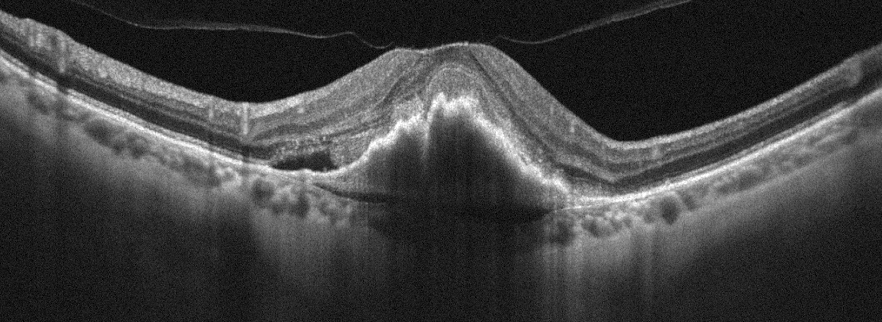

Retinal OCT B-scan
This B-scan demonstrates age-related macular degeneration.